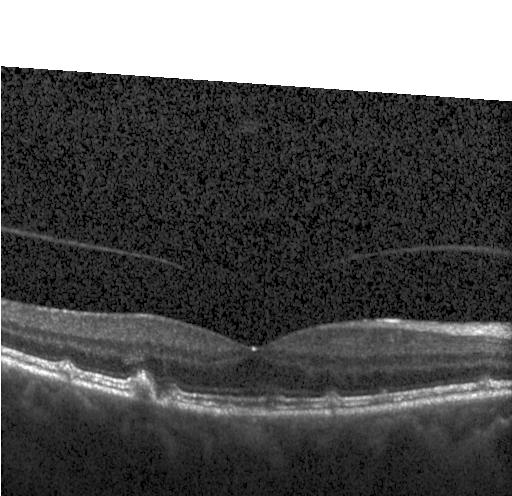

Diagnosis: multiple drusen.